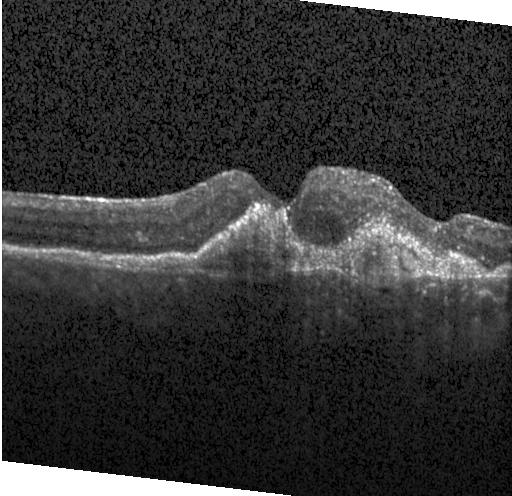
Optical coherence tomography scan. OCT finding: a choroidal neovascular membrane.